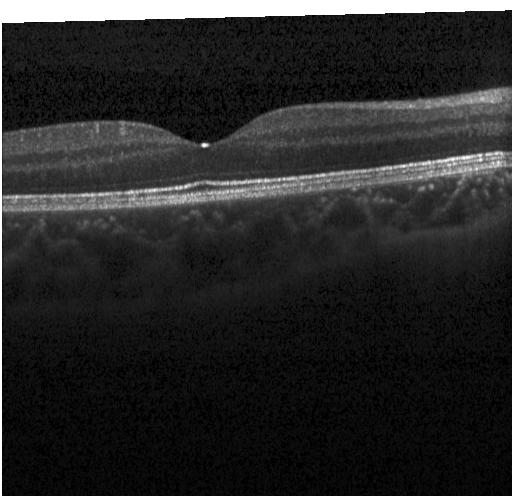

Impression: no CNV, DME, or drusen.